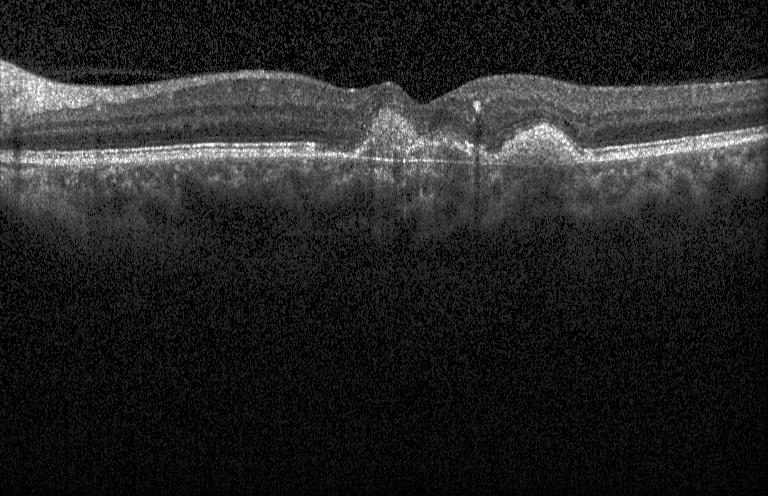

Macular OCT demonstrating choroidal neovascularization (CNV).